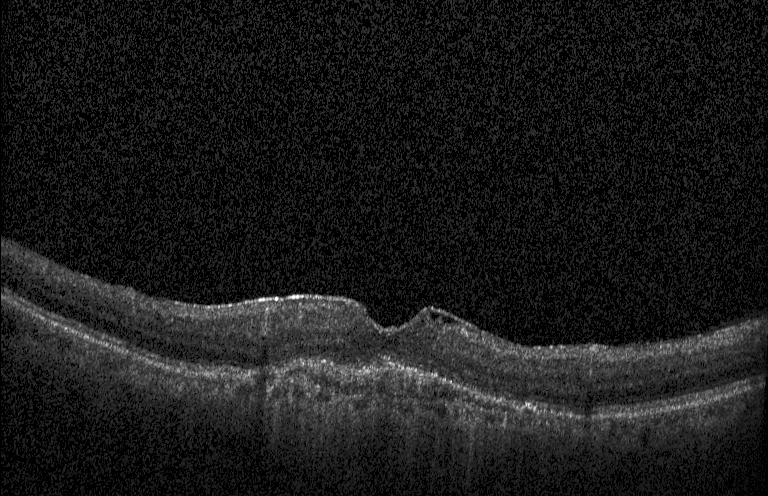
Heidelberg Spectralis · macular scan · SD-OCT · OCT B-scan.
Diagnosis: choroidal neovascularization.